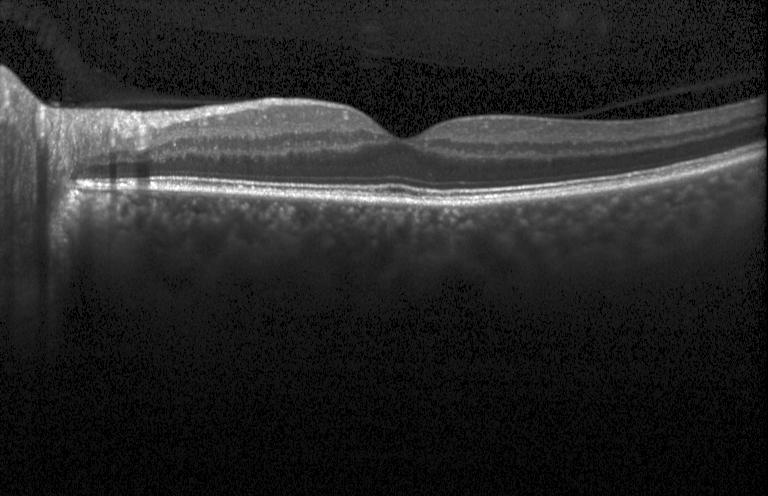 The scan shows no evidence of CNV, DME, or drusen.